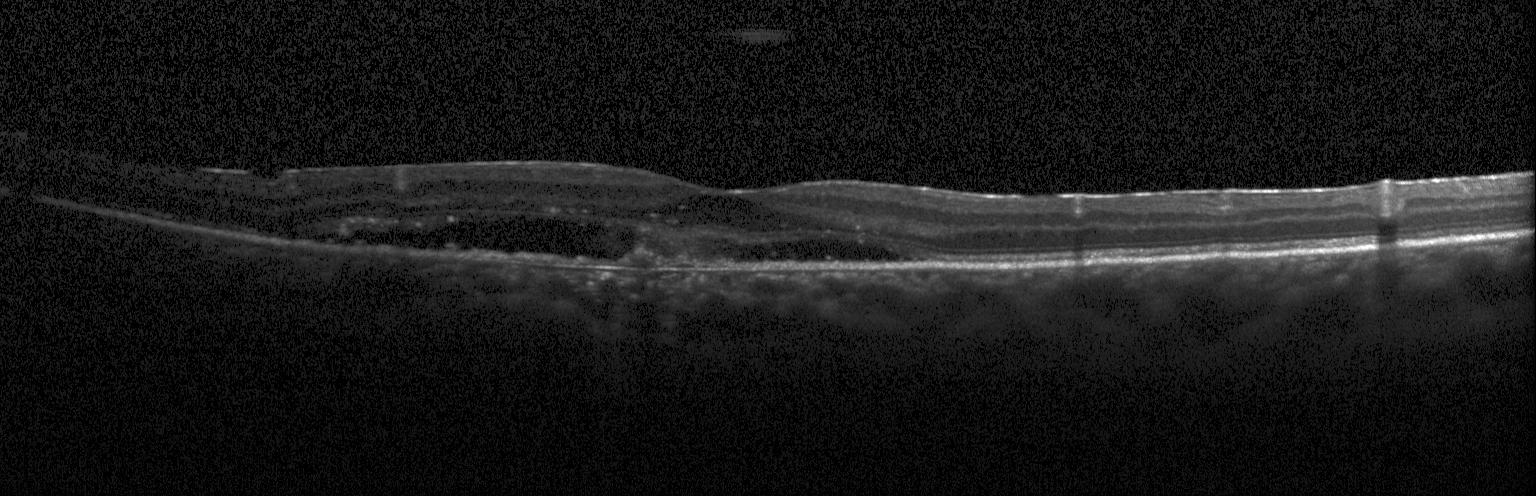 Spectral-domain OCT B-scan: CNV.